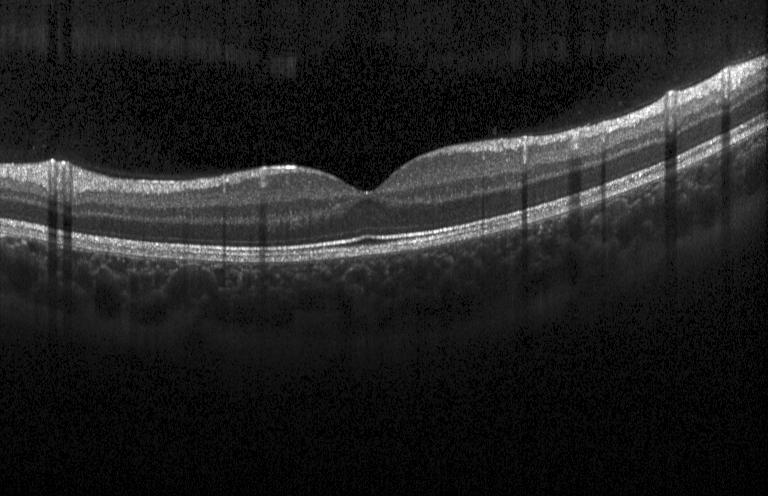

No choroidal neovascularization, no diabetic macular edema, and no drusen.